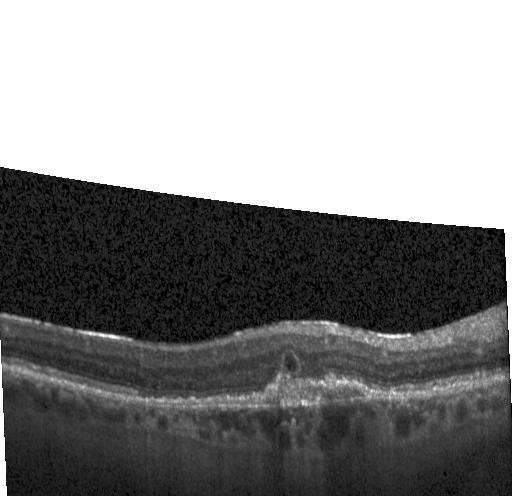
Impression: a choroidal neovascular membrane.